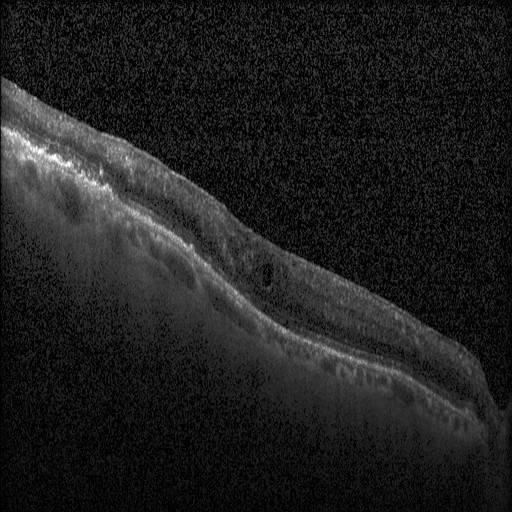
Retinal OCT B-scan — Finding: diabetic macular edema (DME).